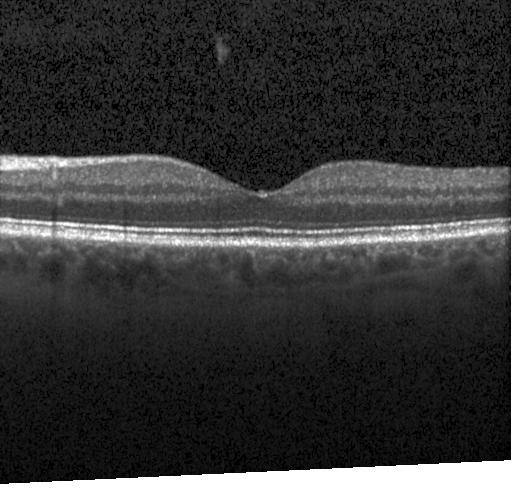

Optical coherence tomography scan — Impression: no evidence of choroidal neovascularization, diabetic macular edema, or drusen.